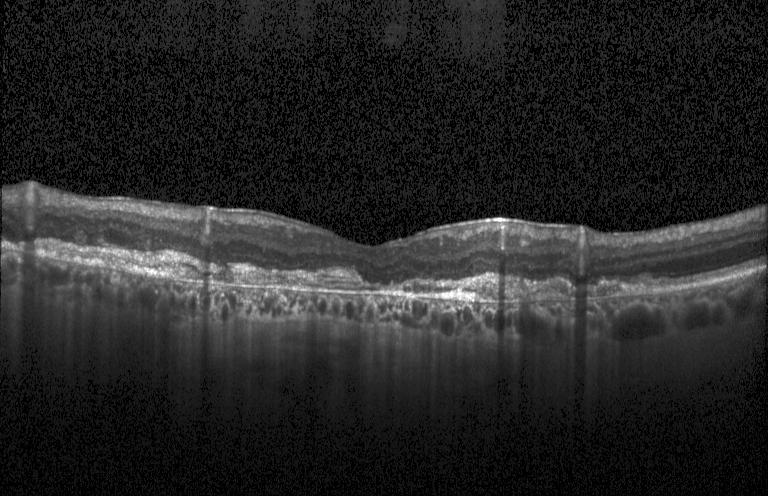

Through the macula. Spectral-domain optical coherence tomography. Heidelberg Spectralis OCT system. Retinal OCT cross-section.
Assessment: choroidal neovascularization.